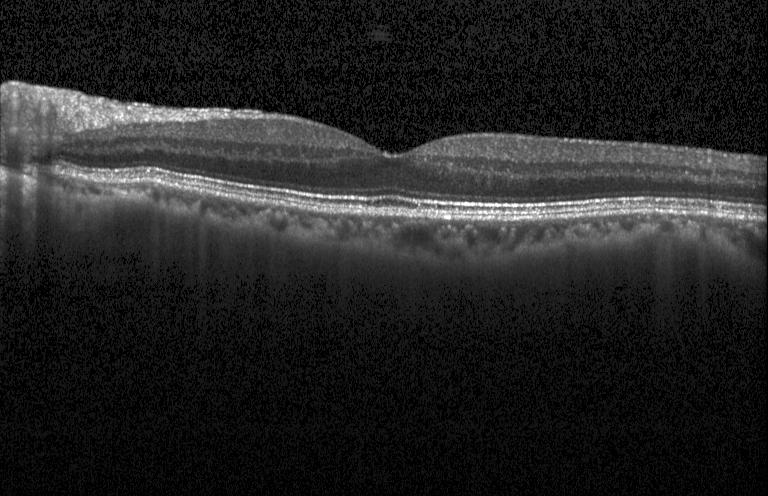 Impression: no choroidal neovascularization, diabetic macular edema, or drusen.